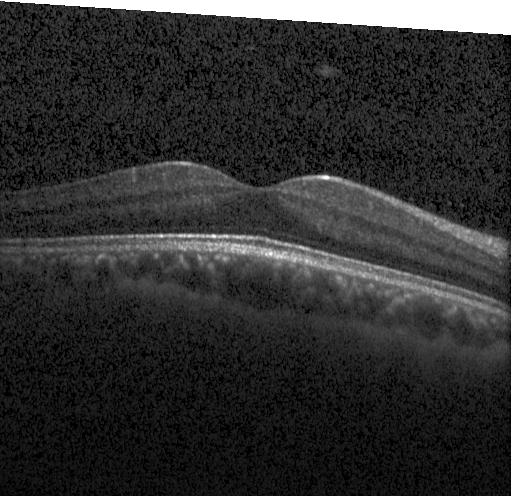

Spectral-domain OCT B-scan: no evidence of CNV, DME, or drusen.